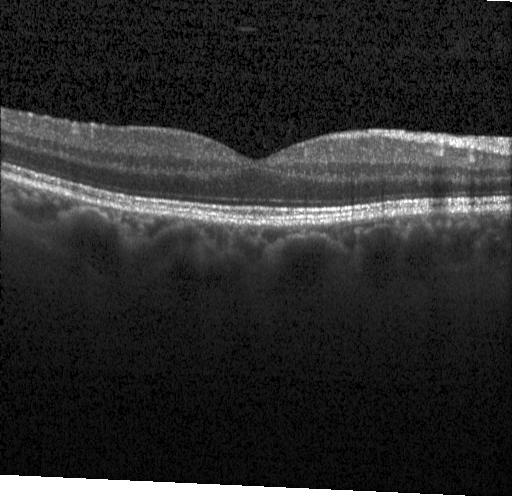

Diagnosis: no evidence of CNV, DME, or drusen.